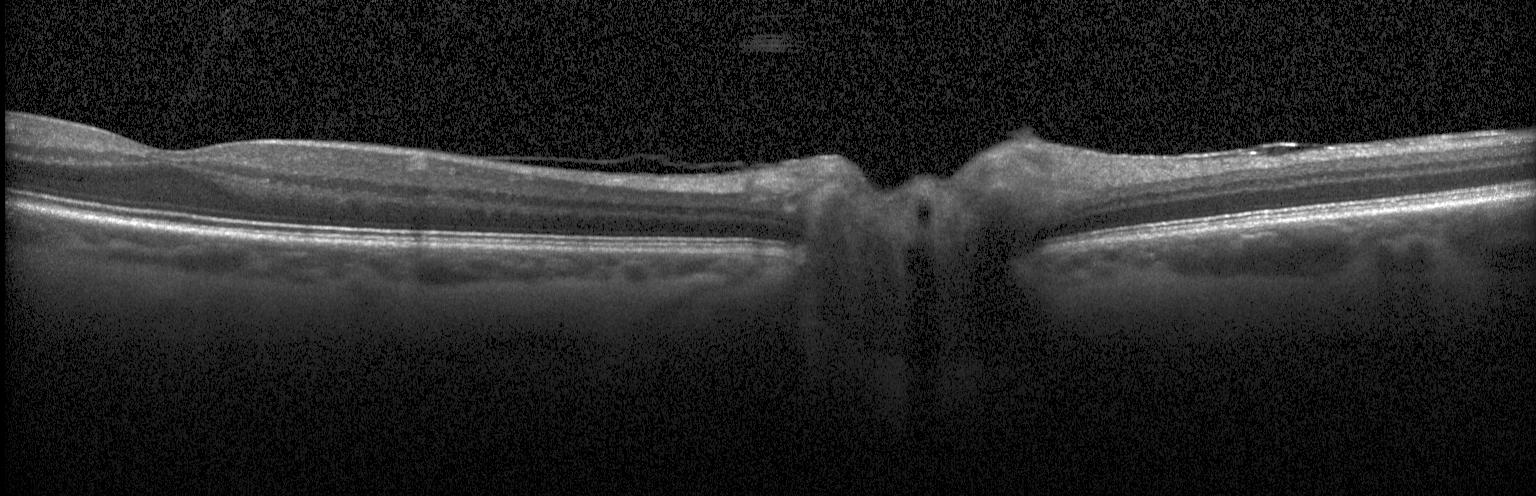 Optical coherence tomography scan · horizontal scan through the fovea — Impression: neither choroidal neovascularization, diabetic macular edema, nor drusen.